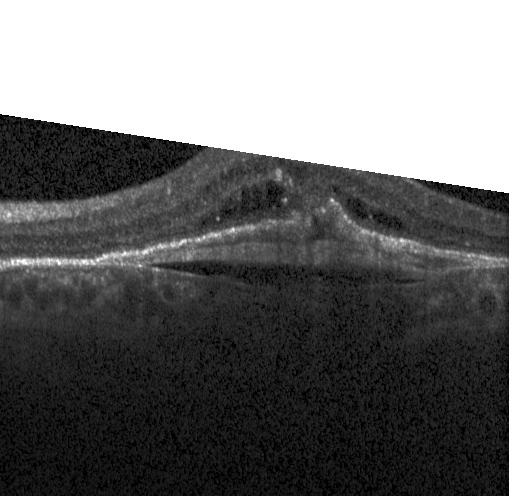
OCT finding: a choroidal neovascular membrane.